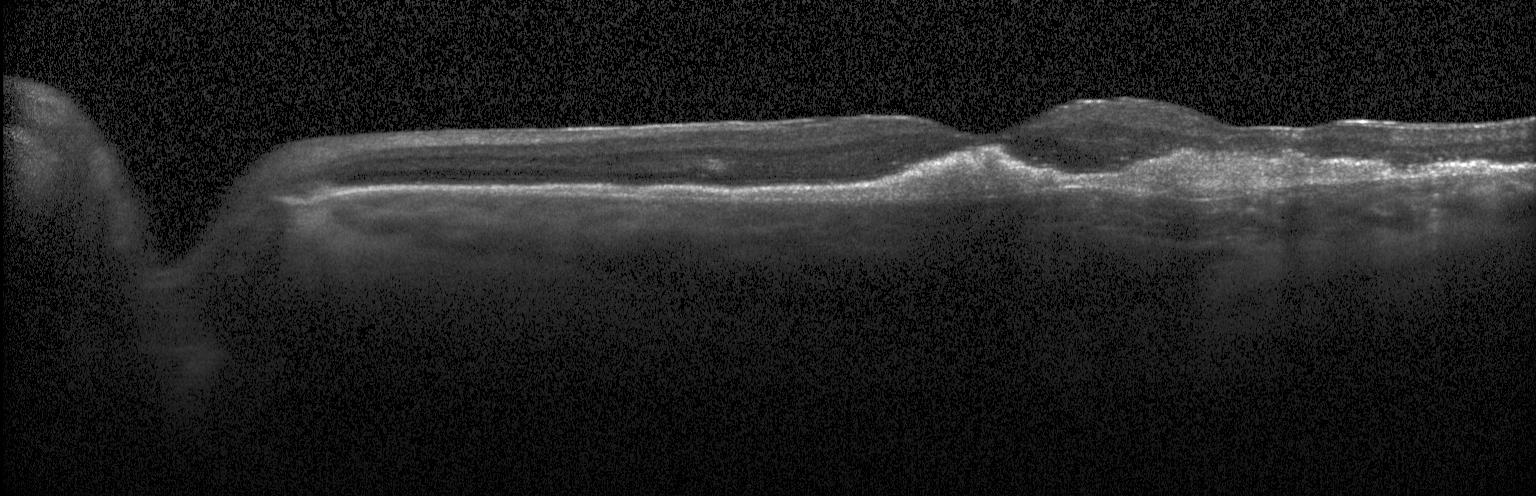
Optical coherence tomography B-scan, SD-OCT. Impression: CNV.